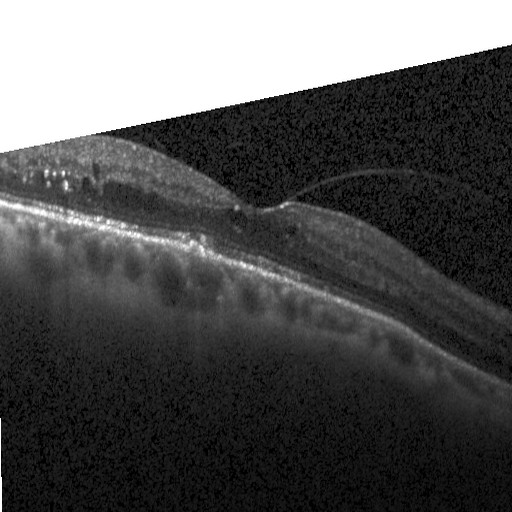

DME.